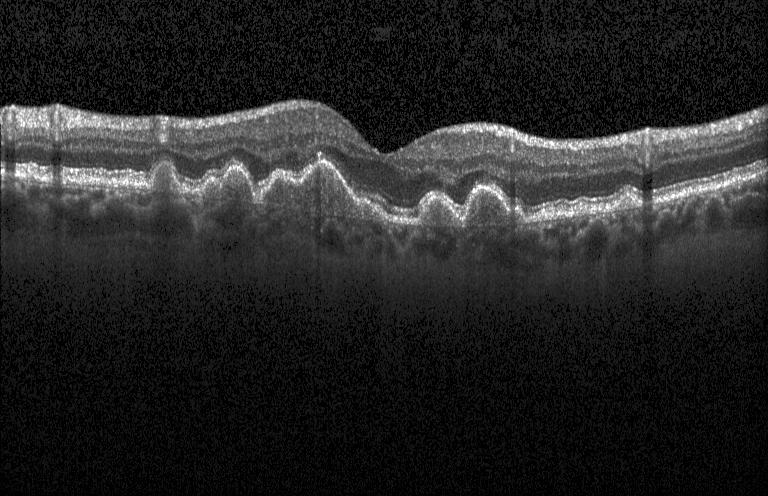 Impression: sub-RPE drusenoid deposits.